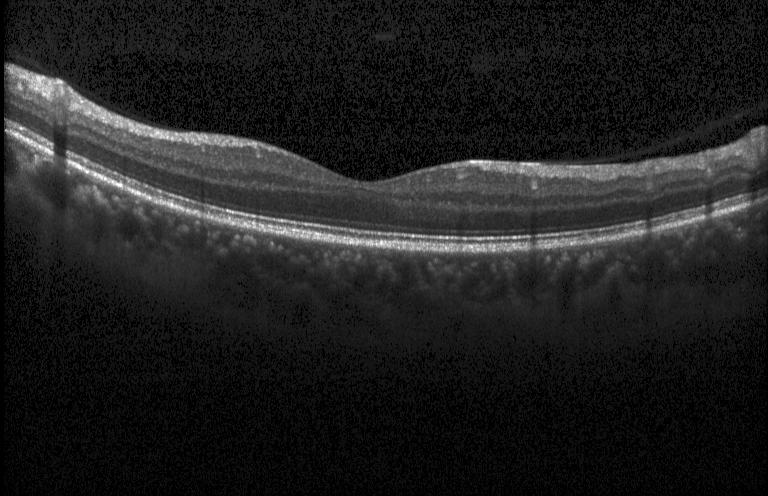 Macular OCT: neither choroidal neovascularization, diabetic macular edema, nor drusen.